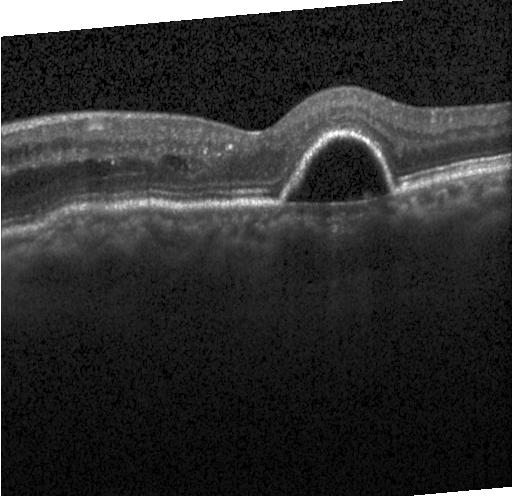 Spectral-domain OCT; through the macula; retinal OCT cross-section — Finding: a choroidal neovascular membrane.